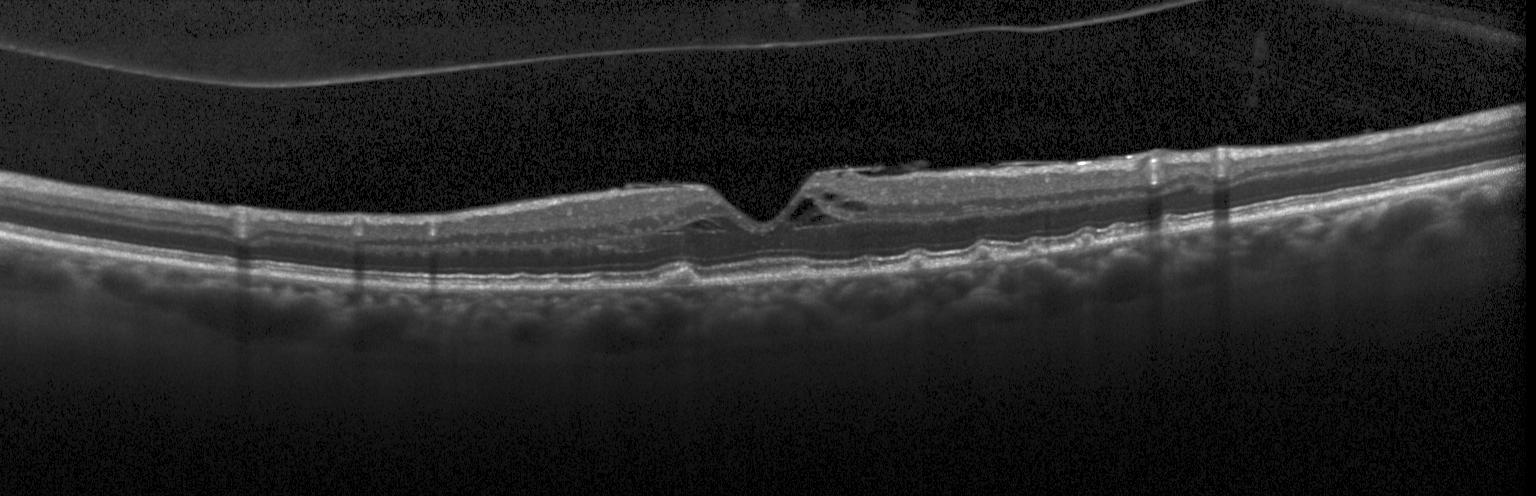 OCT B-scan, centered on the fovea, Heidelberg Spectralis, spectral-domain optical coherence tomography. Impression: sub-RPE drusenoid deposits.